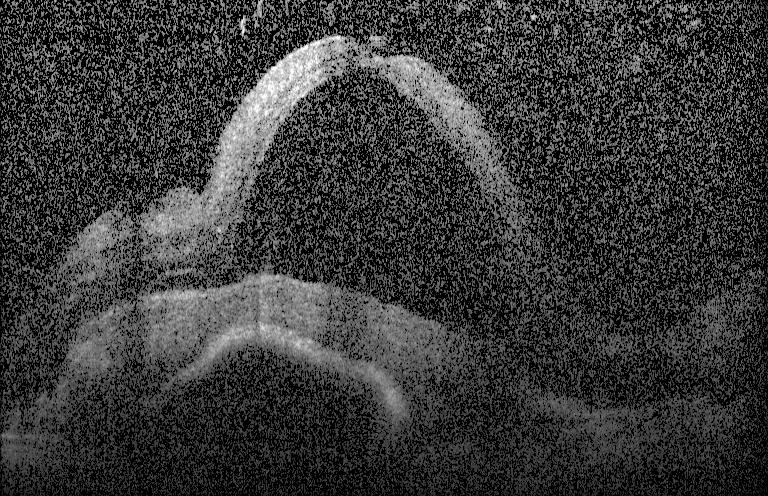

Retinal OCT B-scan; instrument: Heidelberg Spectralis; horizontal scan through the fovea; spectral-domain optical coherence tomography — Diagnosis: a choroidal neovascular membrane.